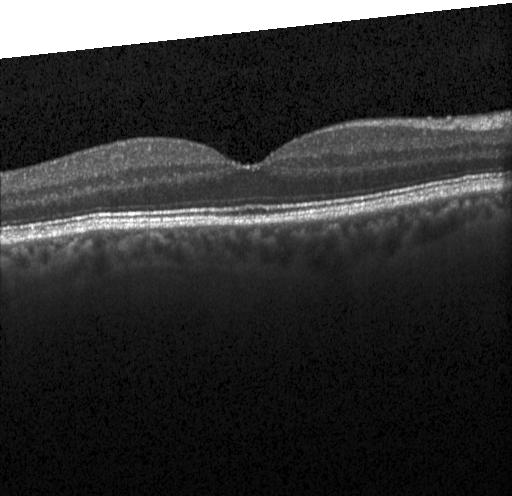
Optical coherence tomography scan
Finding: no evidence of choroidal neovascularization, diabetic macular edema, or drusen.